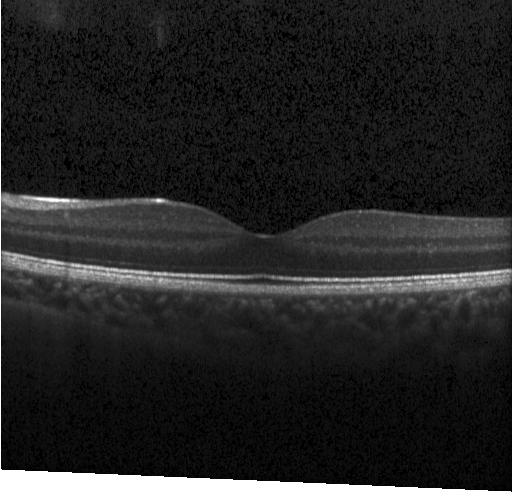

Optical coherence tomography B-scan · instrument: Heidelberg Spectralis · centered on the fovea. Finding: no choroidal neovascularization, diabetic macular edema, or drusen.